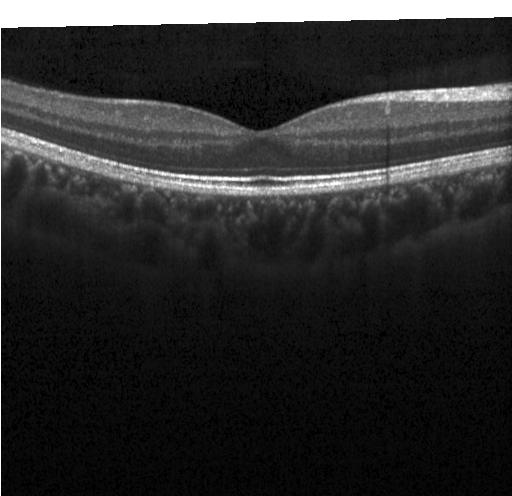

Macular OCT: no choroidal neovascularization, no diabetic macular edema, and no drusen.